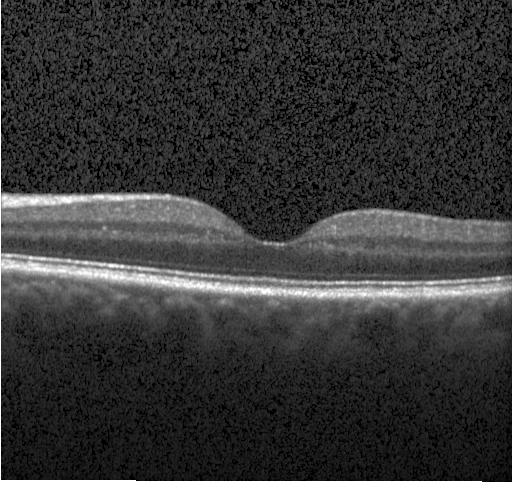
Finding: no choroidal neovascularization, diabetic macular edema, or drusen.